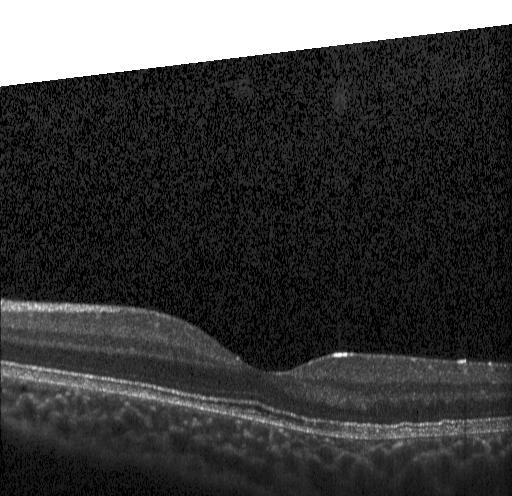 Heidelberg Spectralis. Optical coherence tomography B-scan. Finding: neither choroidal neovascularization, diabetic macular edema, nor drusen.